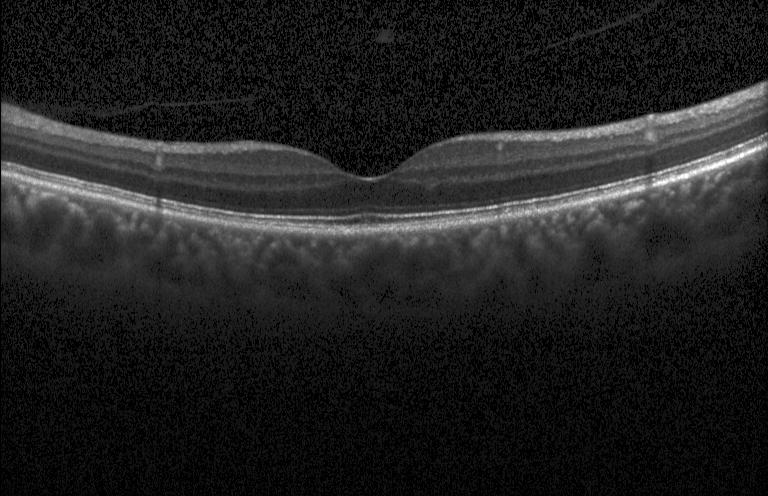

Retinal OCT cross-section; spectral-domain optical coherence tomography.
Diagnosis: no evidence of CNV, DME, or drusen.